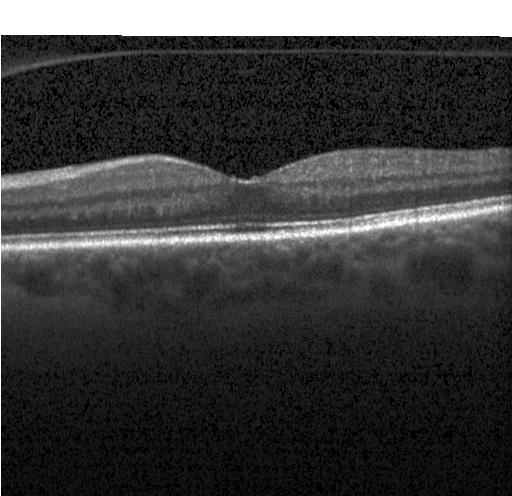 Instrument: Heidelberg Spectralis, optical coherence tomography B-scan, through the macula, SD-OCT. OCT finding: no evidence of choroidal neovascularization, diabetic macular edema, or drusen.